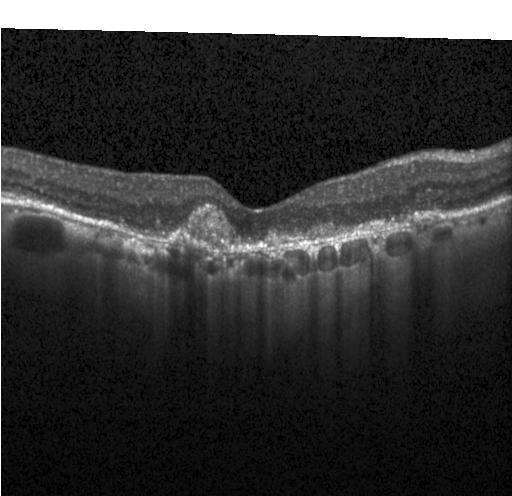
SD-OCT. Optical coherence tomography scan. Centered on the fovea. Heidelberg Spectralis — Finding: a choroidal neovascular membrane.